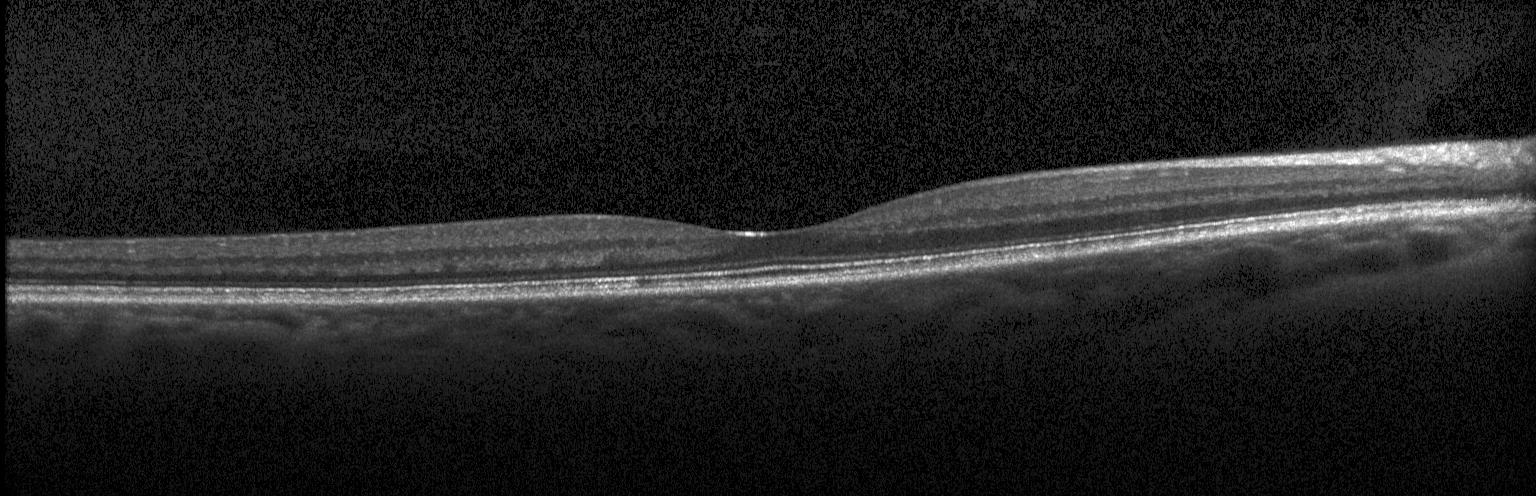 OCT B-scan showing no evidence of choroidal neovascularization, diabetic macular edema, or drusen.